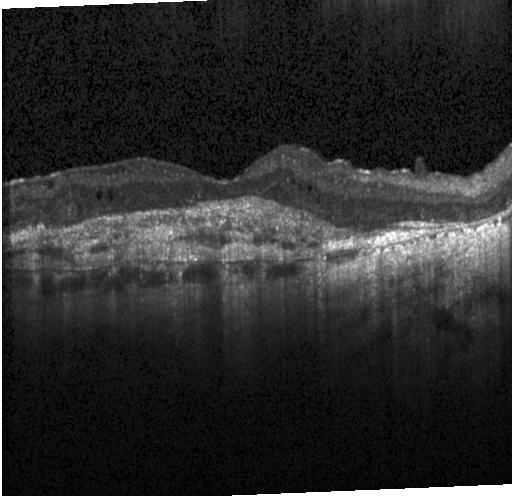

Acquired on a Heidelberg Spectralis, macular scan, SD-OCT, optical coherence tomography scan. Impression: a choroidal neovascular membrane.